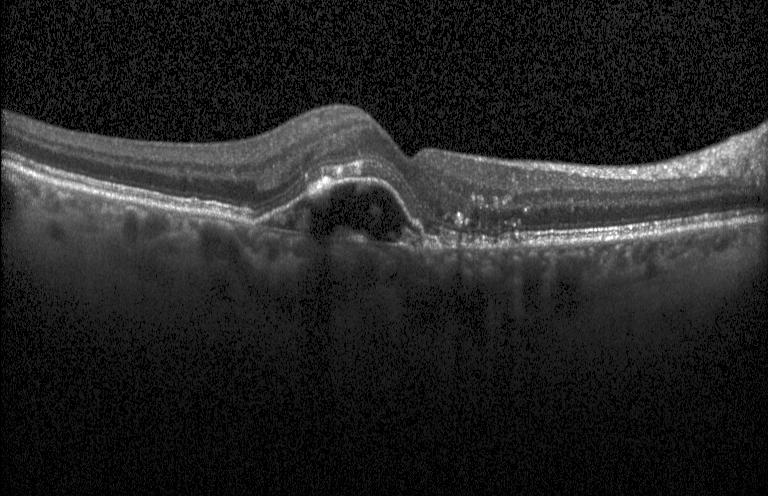

Optical coherence tomography B-scan — Impression: choroidal neovascularization.